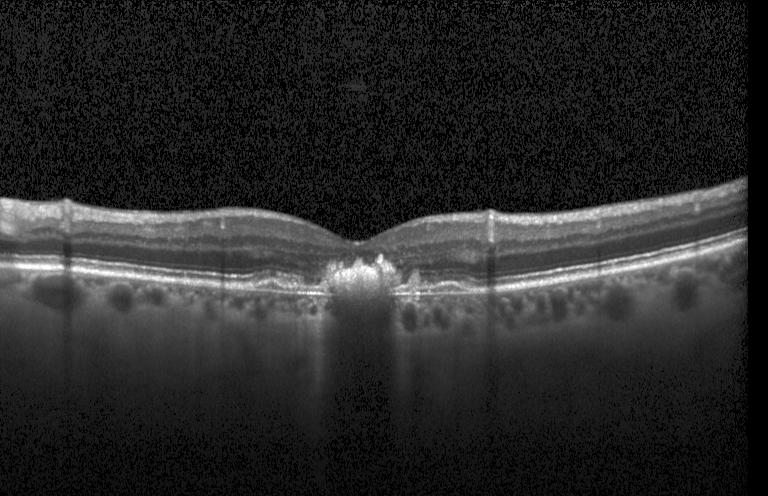
Fovea-centered · optical coherence tomography scan — Impression: a choroidal neovascular membrane.